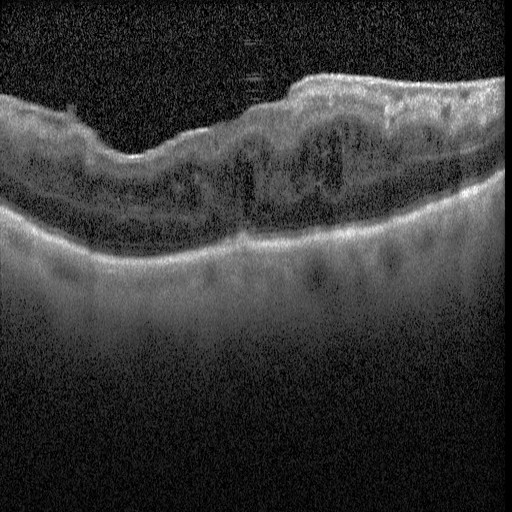

Instrument: Heidelberg Spectralis; through the macula; optical coherence tomography scan.
The scan shows diabetic macular edema.